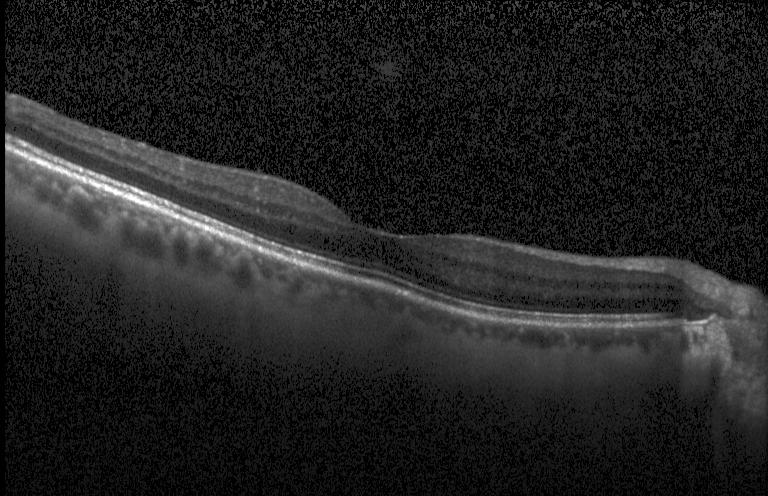 Retinal OCT cross-section showing no evidence of CNV, DME, or drusen.